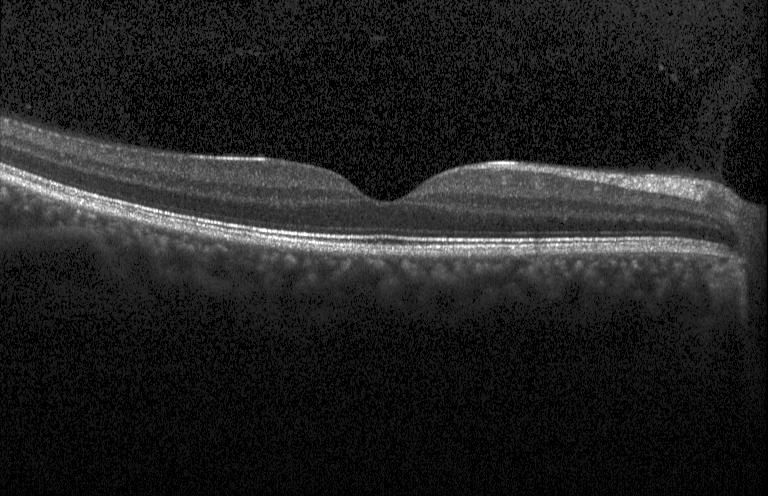

No CNV, DME, or drusen.